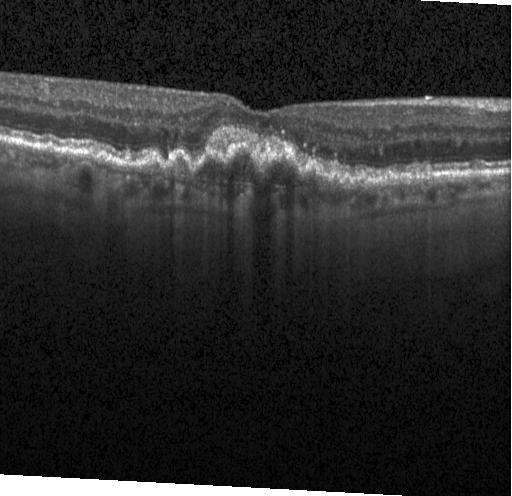 Spectral-domain optical coherence tomography; centered on the fovea; OCT line scan.
This B-scan demonstrates a choroidal neovascular membrane.